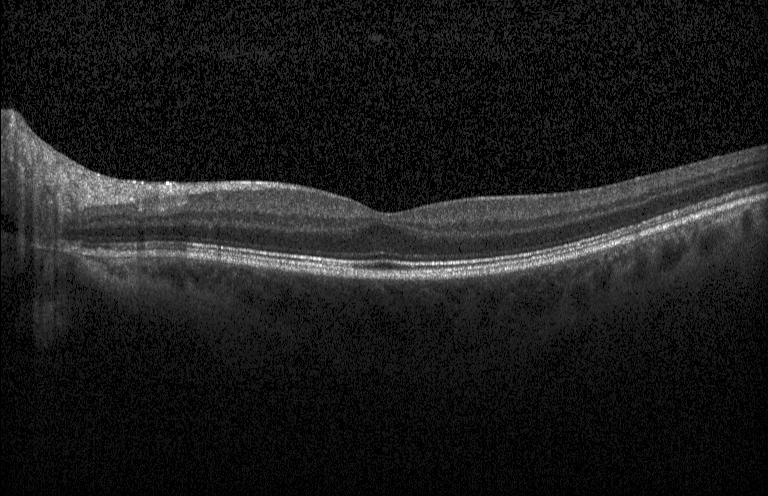
Retinal OCT cross-section · spectral-domain OCT · through the macula · instrument: Heidelberg Spectralis
Assessment: no CNV, no DME, and no drusen.